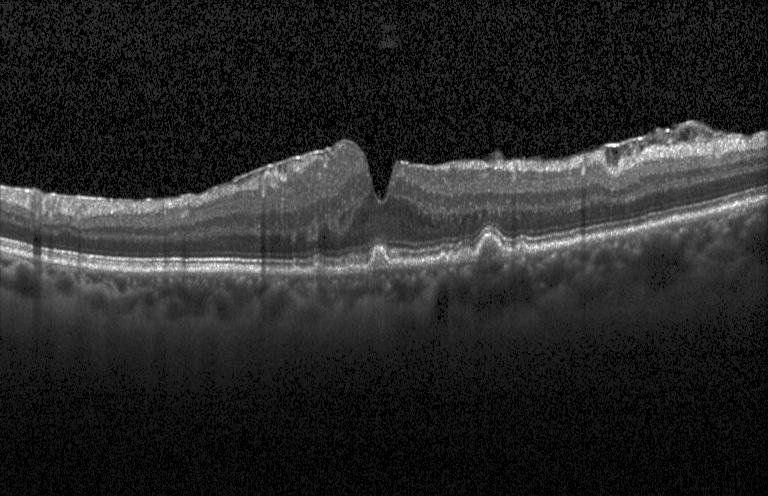

Instrument: Heidelberg Spectralis. Optical coherence tomography scan. Finding: drusen.